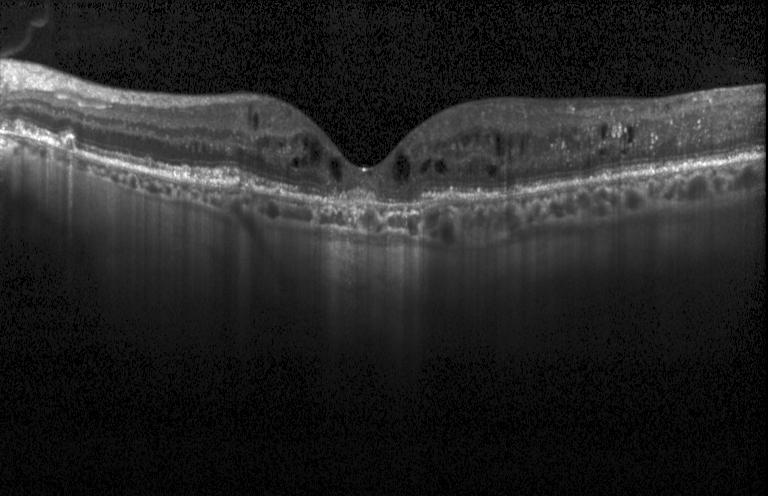 SD-OCT · Heidelberg Spectralis · optical coherence tomography scan · fovea-centered.
Diagnosis: a choroidal neovascular membrane.